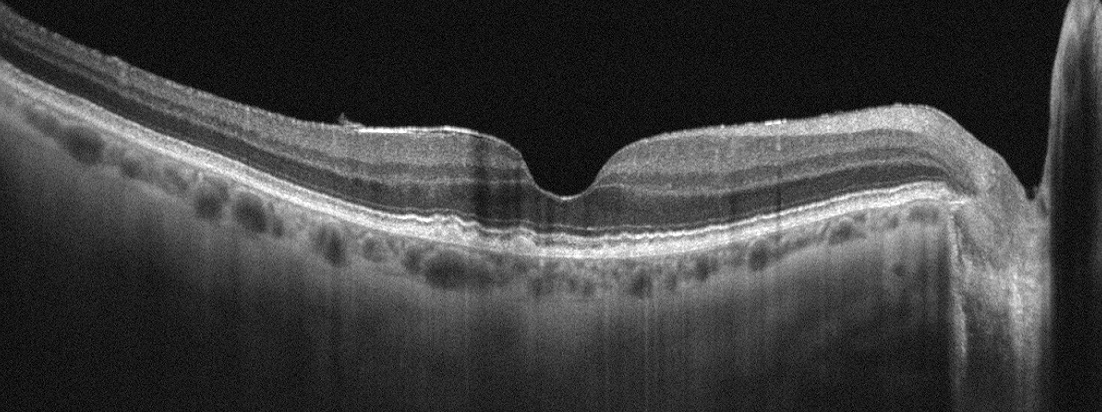 Through the macula; instrument: Optovue Avanti RTVue XR; retinal OCT B-scan — Impression: epiretinal membrane.